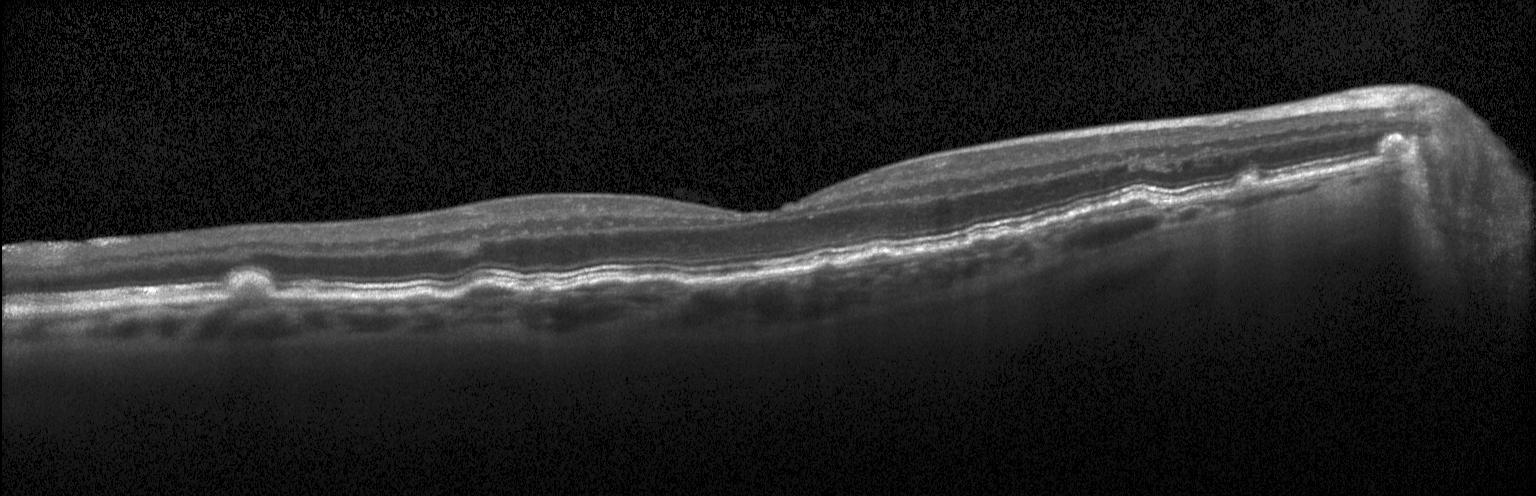

Diagnosis: drusen.